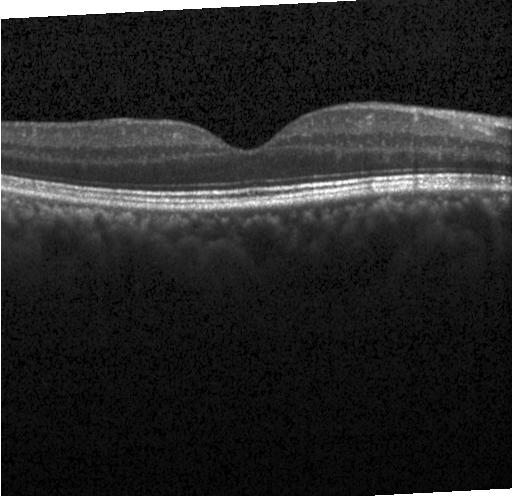 Dx: no CNV, DME, or drusen.